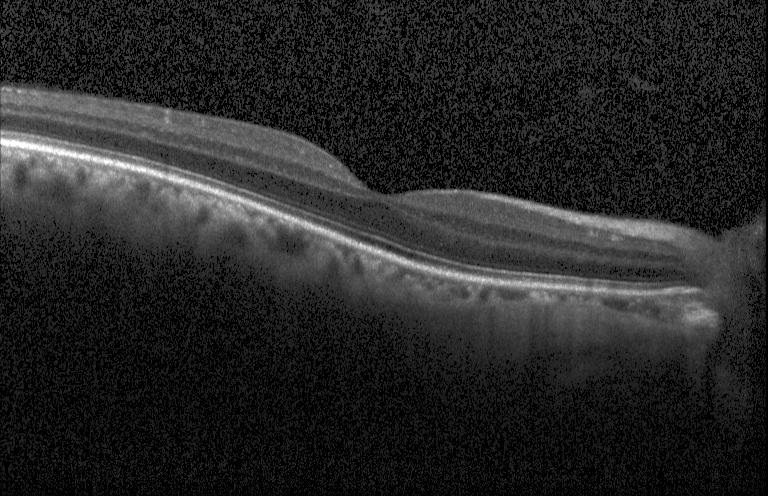 Retinal OCT cross-section showing no CNV, no DME, and no drusen.